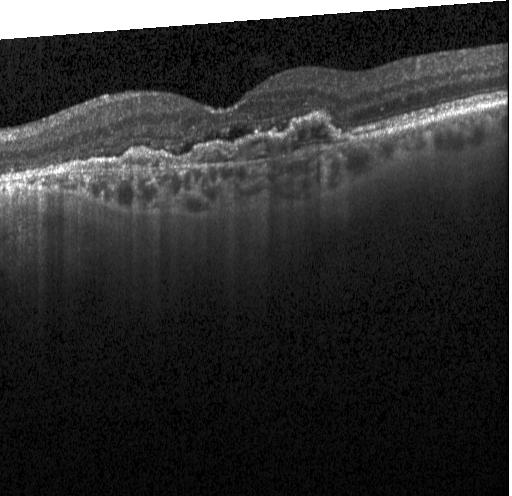 Diagnosis: choroidal neovascularization (CNV).